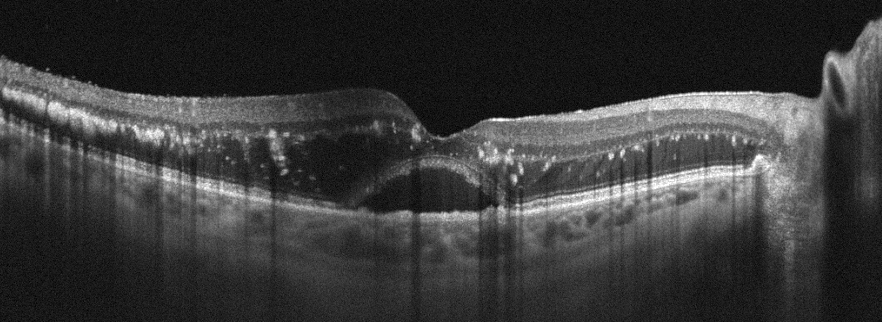 Macular scan · acquired on an Optovue Avanti RTVue XR · OCT B-scan — Diagnosis: retinal vein occlusion.